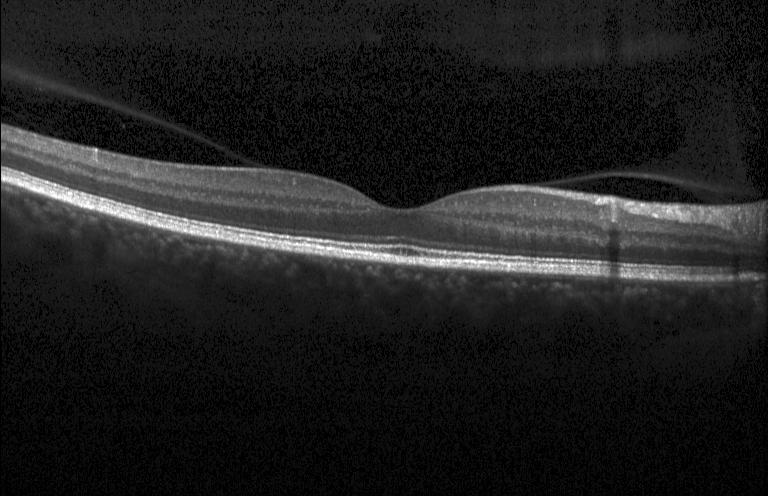 Dx: no choroidal neovascularization, diabetic macular edema, or drusen.